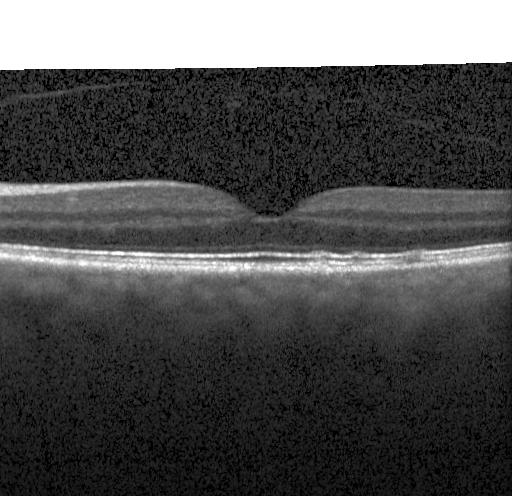 Heidelberg Spectralis OCT system · spectral-domain optical coherence tomography · OCT B-scan — Finding: neither choroidal neovascularization, diabetic macular edema, nor drusen.